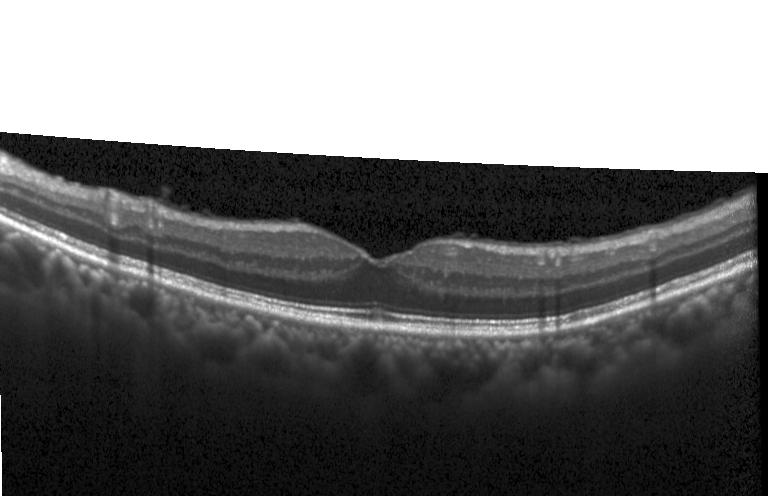 Horizontal scan through the fovea, spectral-domain optical coherence tomography, optical coherence tomography scan, acquired on a Heidelberg Spectralis
Diagnosis: no CNV, no DME, and no drusen.